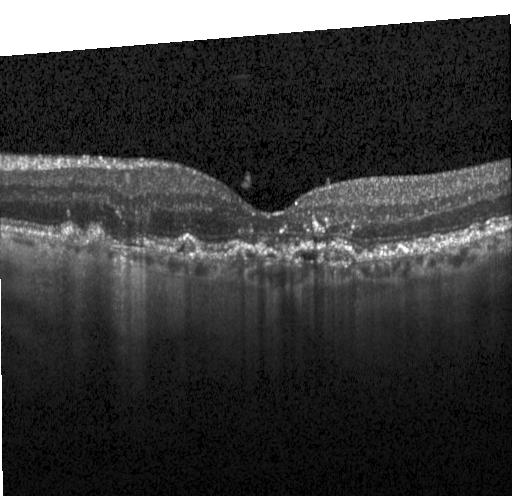 Macular OCT: CNV.